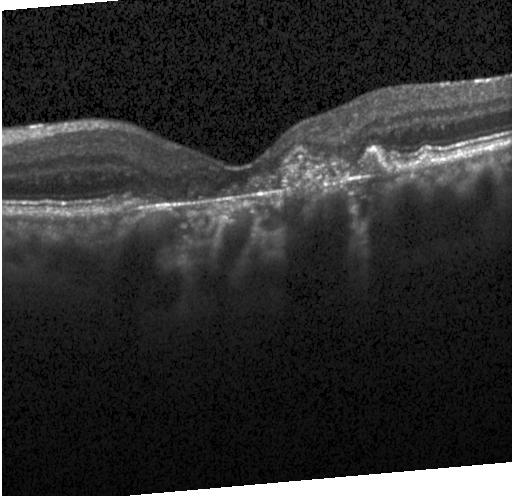 Retinal OCT B-scan
Impression: choroidal neovascularization (CNV).